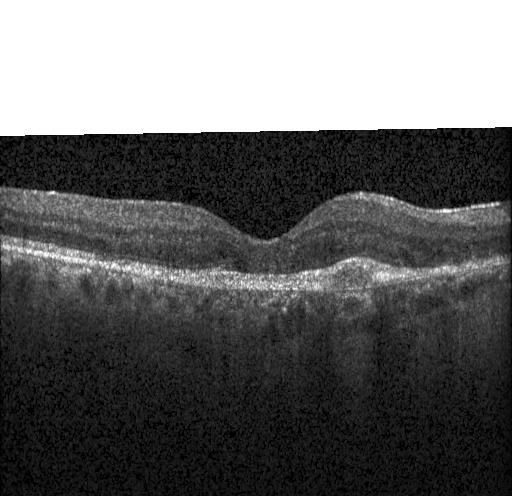

Macular OCT: choroidal neovascularization (CNV).